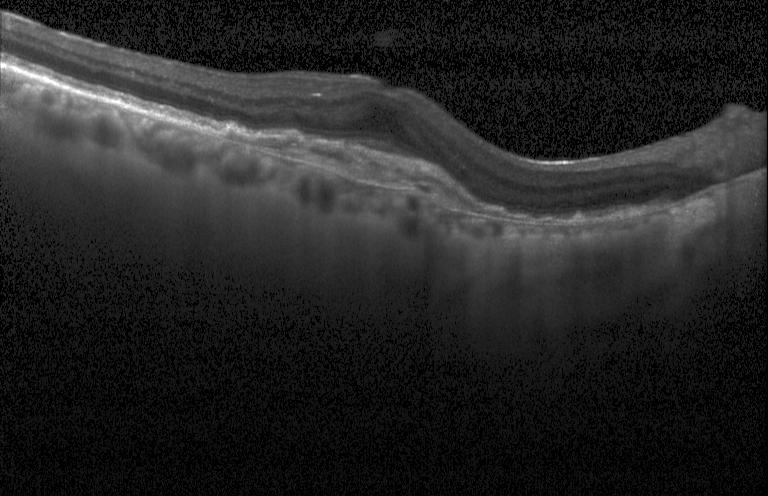 OCT B-scan — Finding: choroidal neovascularization.